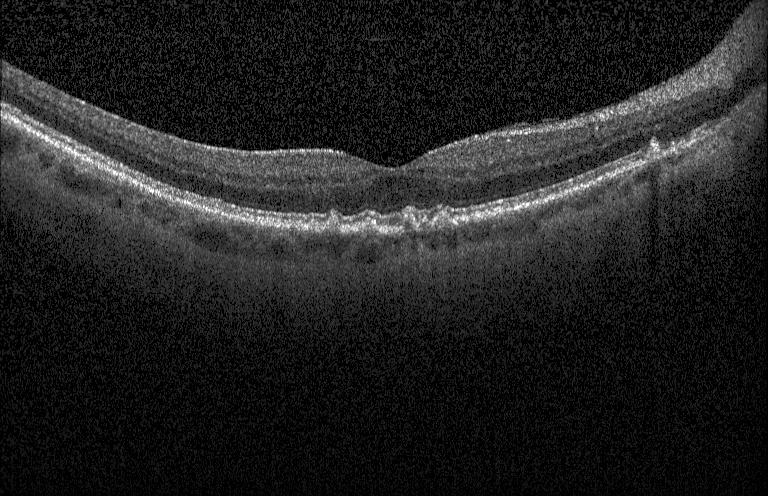

Finding: drusen.